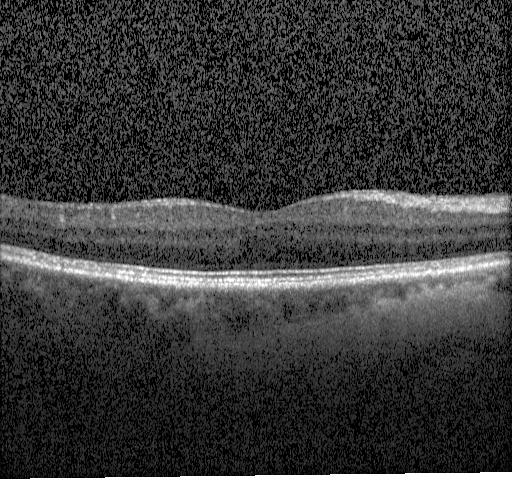 Spectral-domain OCT; fovea-centered; retinal OCT B-scan.
Impression: no evidence of choroidal neovascularization, diabetic macular edema, or drusen.